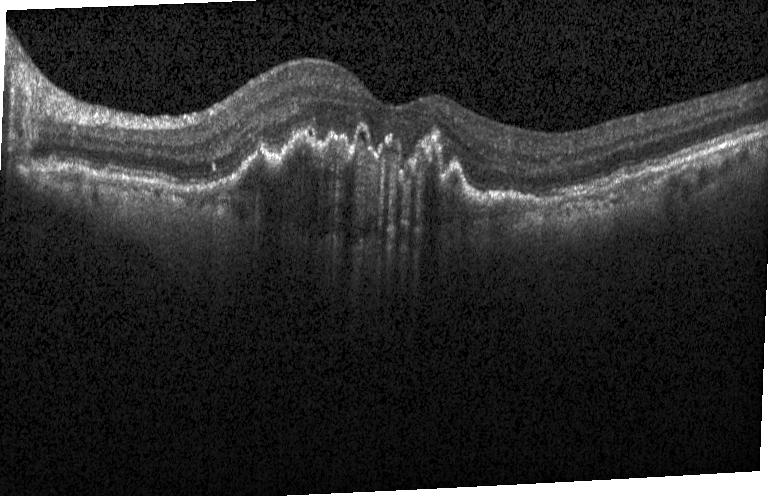 Heidelberg Spectralis, retinal OCT cross-section, horizontal scan through the fovea. Finding: choroidal neovascularization.